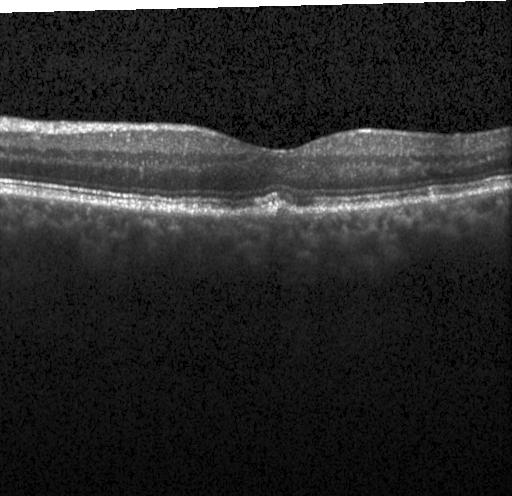
Spectral-domain OCT; instrument: Heidelberg Spectralis; retinal OCT B-scan.
Diagnosis: drusen.